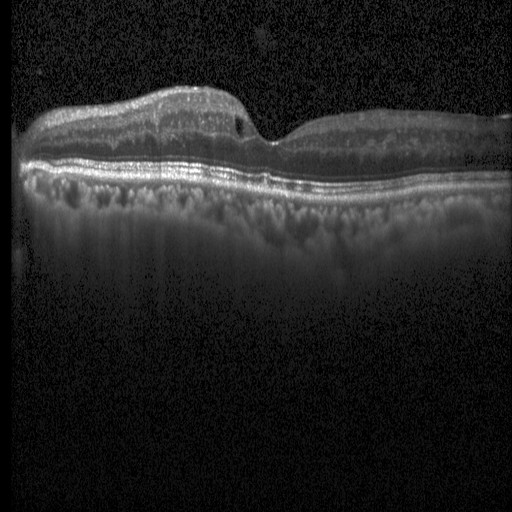 SD-OCT. Fovea-centered. Retinal OCT B-scan. Heidelberg Spectralis — The scan shows diabetic macular edema.